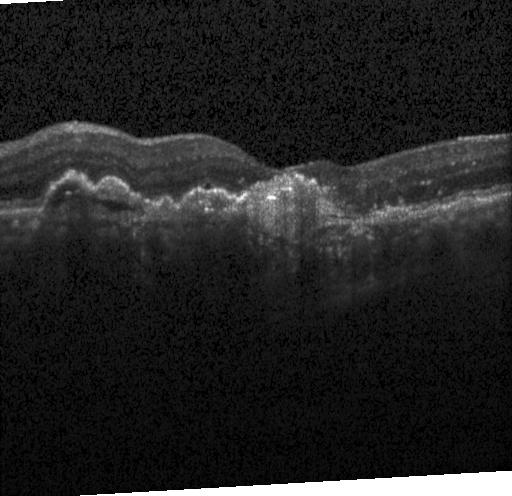

Spectral-domain OCT. Centered on the fovea. Acquired on a Heidelberg Spectralis. Optical coherence tomography B-scan. This B-scan demonstrates choroidal neovascularization (CNV).